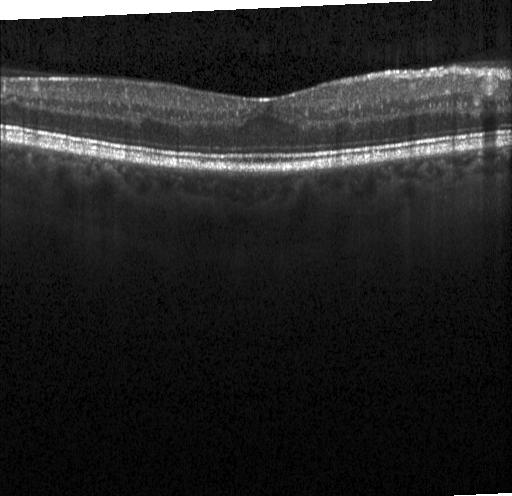 Optical coherence tomography B-scan.
Diagnosis: neither CNV, DME, nor drusen.